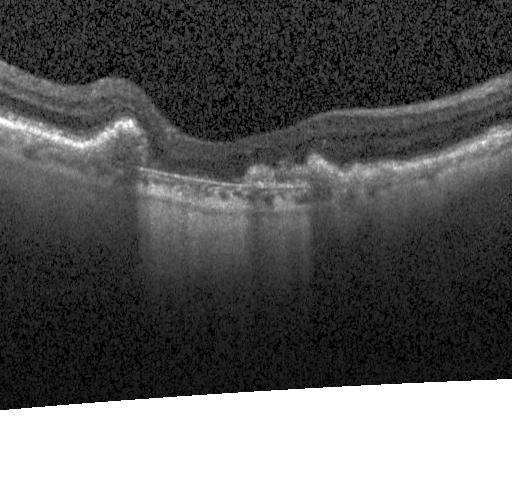 Dx: a choroidal neovascular membrane.